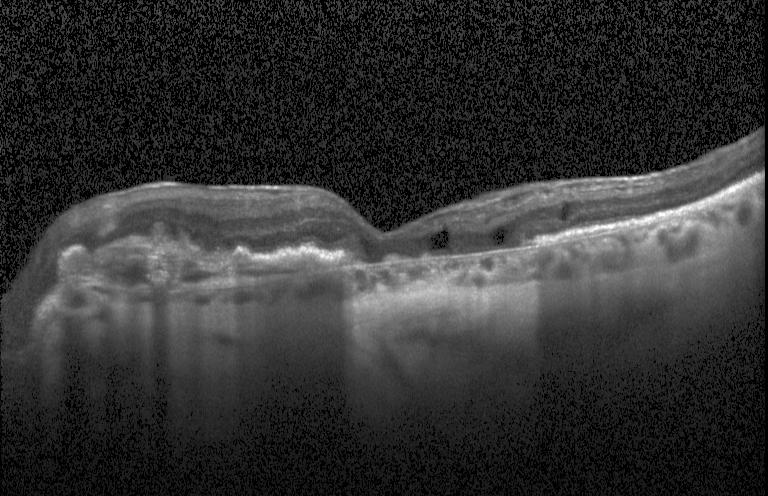

OCT B-scan. SD-OCT. Centered on the fovea. Heidelberg Spectralis. Diagnosis: choroidal neovascularization.